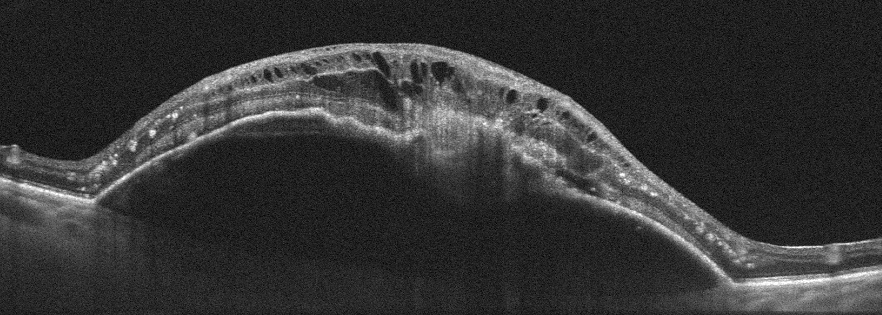
Oculus sinister, OCT line scan. Finding: age-related macular degeneration.